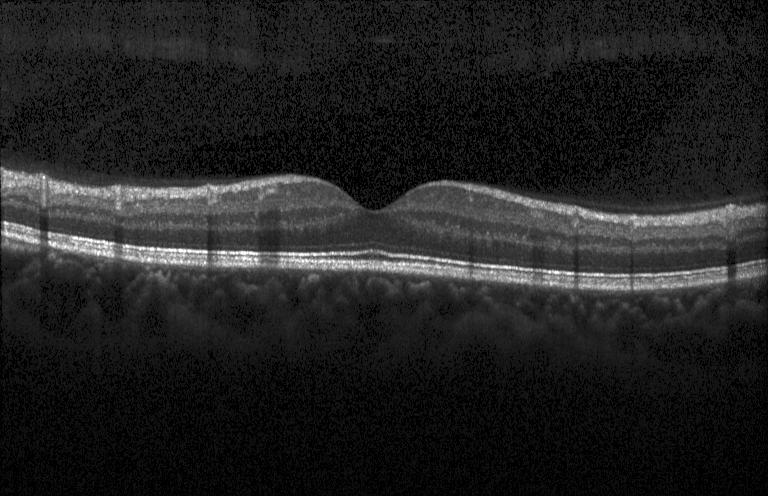

Through the macula, spectral-domain OCT, acquired on a Heidelberg Spectralis, optical coherence tomography scan. No evidence of CNV, DME, or drusen.